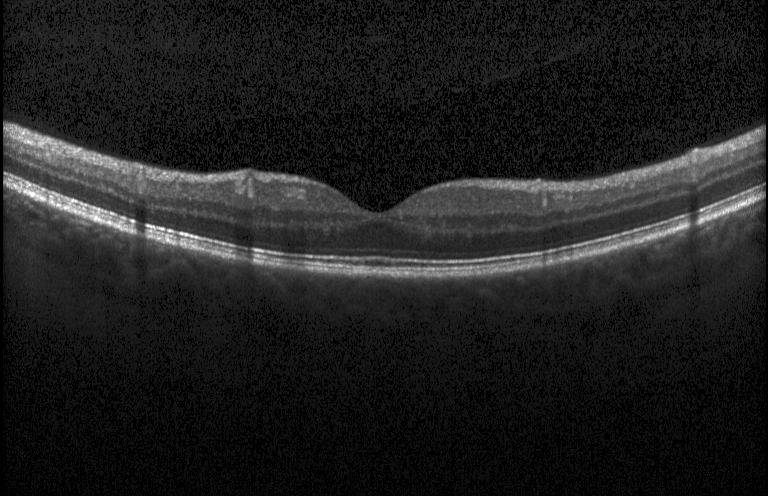 Retinal OCT B-scan · spectral-domain OCT · acquired on a Heidelberg Spectralis
Finding: no CNV, no DME, and no drusen.